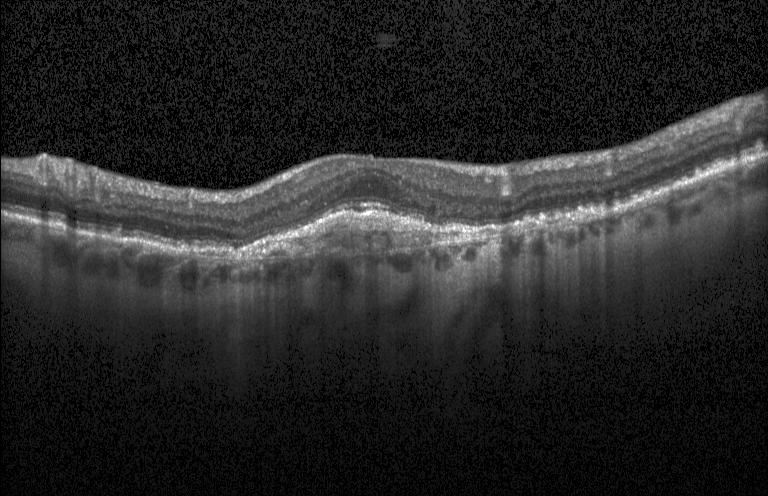 Spectral-domain optical coherence tomography. Acquired on a Heidelberg Spectralis. Optical coherence tomography scan. Macular scan — Dx: choroidal neovascularization (CNV).